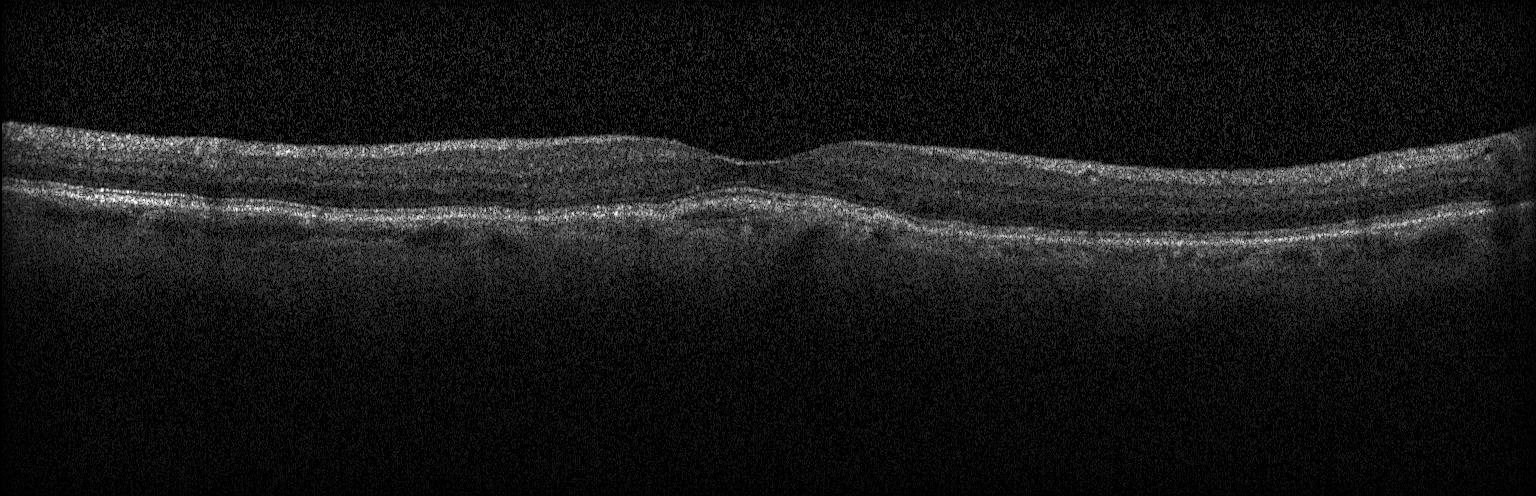

Through the macula, Heidelberg Spectralis OCT system, spectral-domain optical coherence tomography, retinal OCT B-scan — This B-scan demonstrates choroidal neovascularization (CNV).